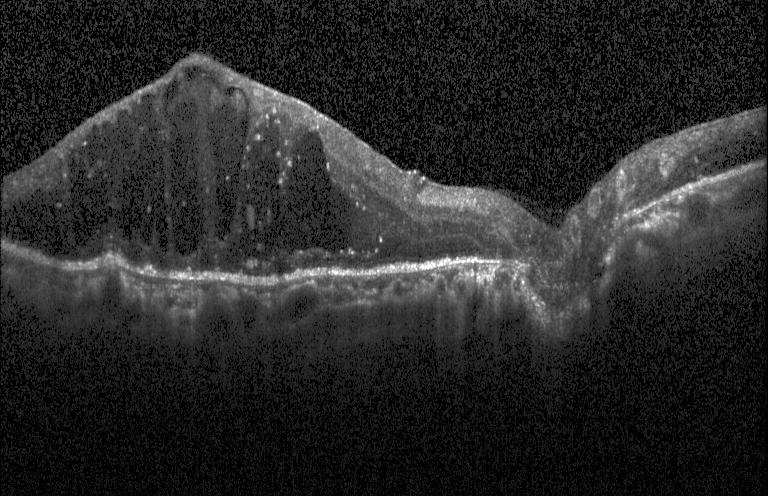 Retinal OCT cross-section · instrument: Heidelberg Spectralis · fovea-centered · SD-OCT.
This B-scan demonstrates diabetic macular edema (DME).